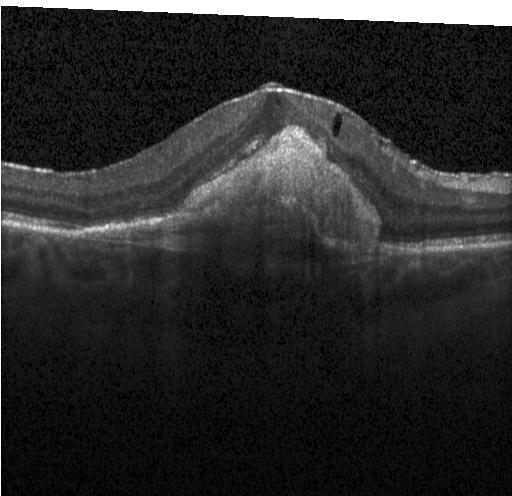

Optical coherence tomography B-scan, Heidelberg Spectralis OCT system
Diagnosis: a choroidal neovascular membrane.